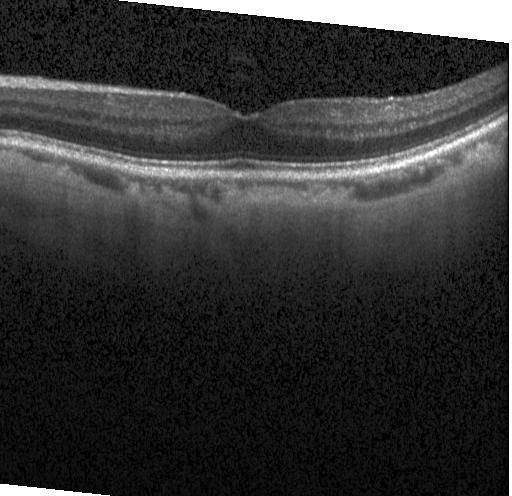

OCT finding: no evidence of choroidal neovascularization, diabetic macular edema, or drusen.